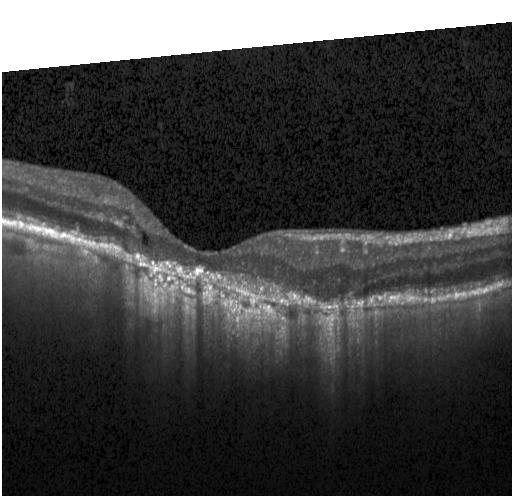
Optical coherence tomography scan
The scan shows CNV.